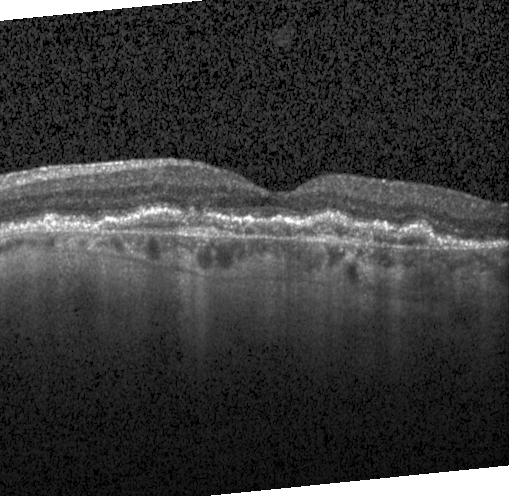

Instrument: Heidelberg Spectralis · spectral-domain OCT · OCT line scan.
The scan shows a choroidal neovascular membrane.